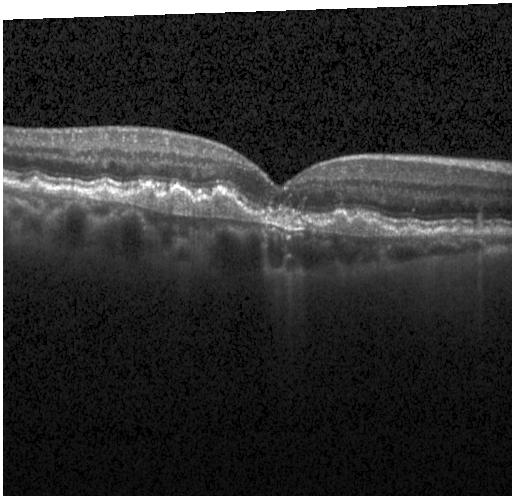 Assessment: a choroidal neovascular membrane.